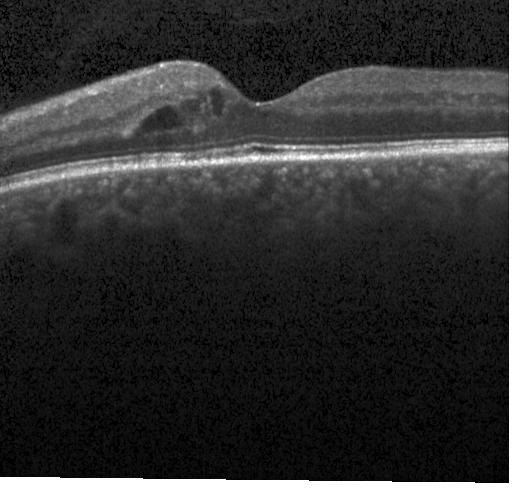
Optical coherence tomography B-scan — Finding: DME.